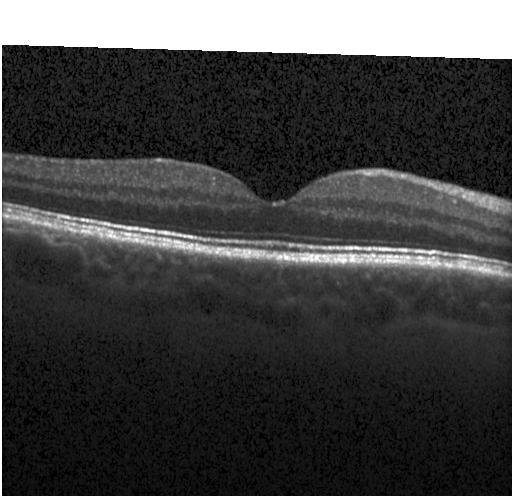

Fovea-centered; OCT B-scan; instrument: Heidelberg Spectralis; spectral-domain OCT
The scan shows no CNV, DME, or drusen.